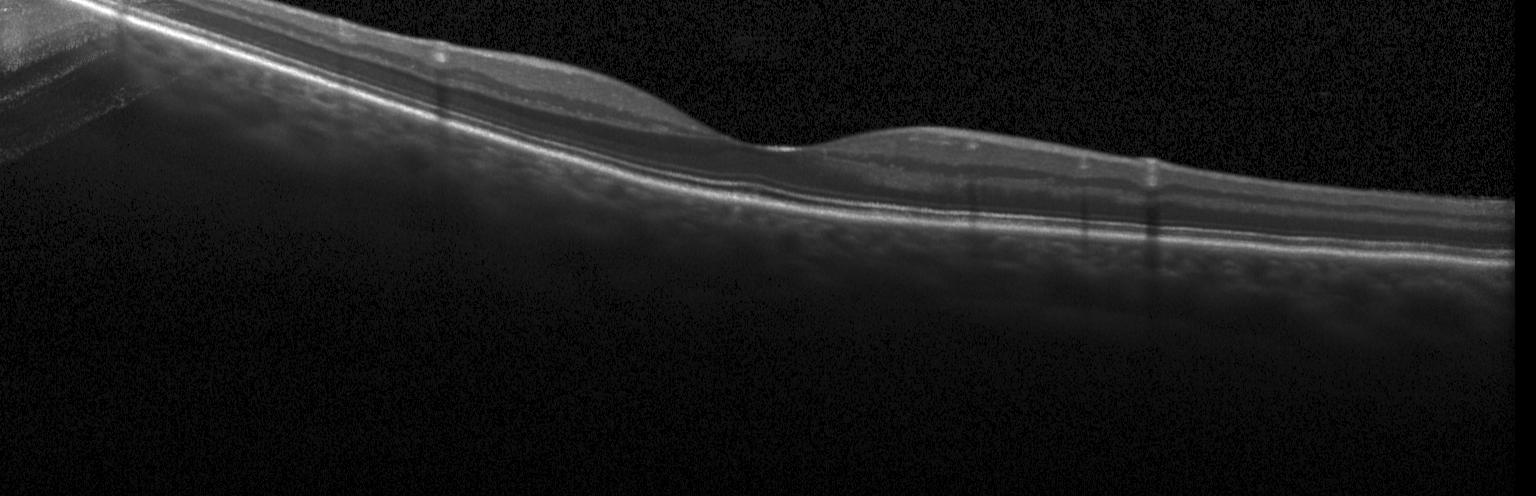

Finding: no evidence of choroidal neovascularization, diabetic macular edema, or drusen.